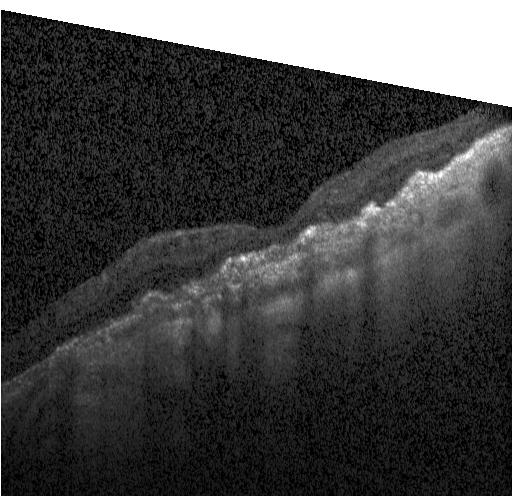
Spectral-domain optical coherence tomography. OCT line scan. Heidelberg Spectralis OCT system.
Finding: a choroidal neovascular membrane.